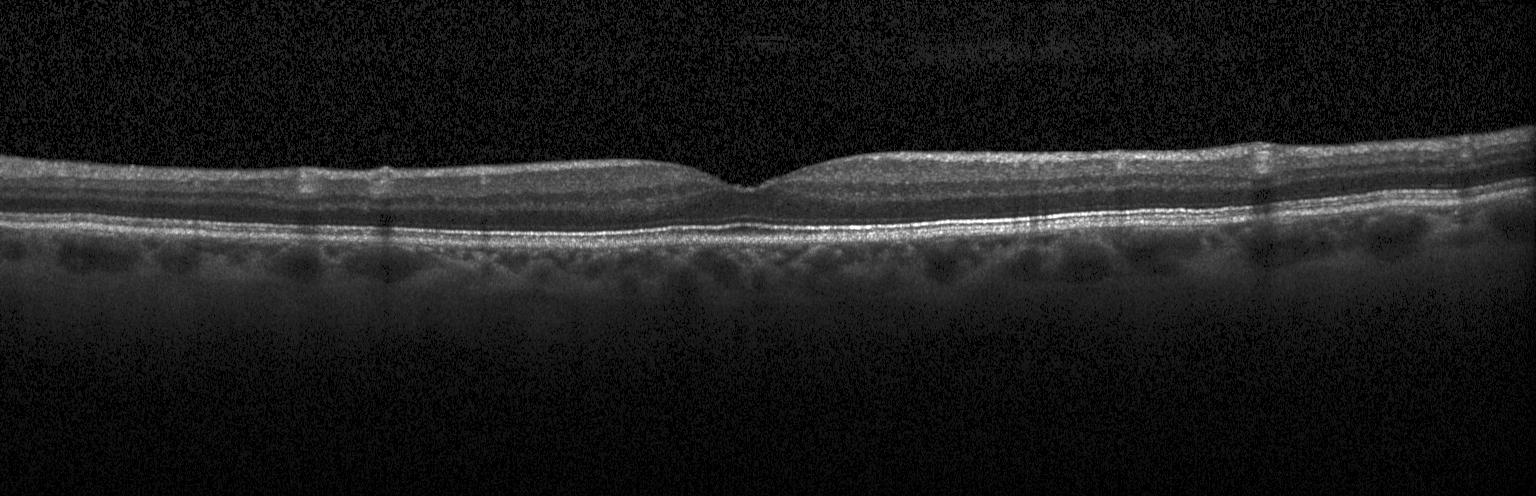
Spectral-domain OCT B-scan: no CNV, no DME, and no drusen.